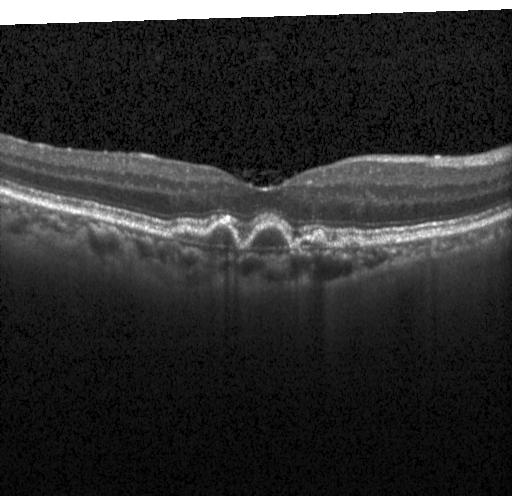 Impression: a choroidal neovascular membrane.